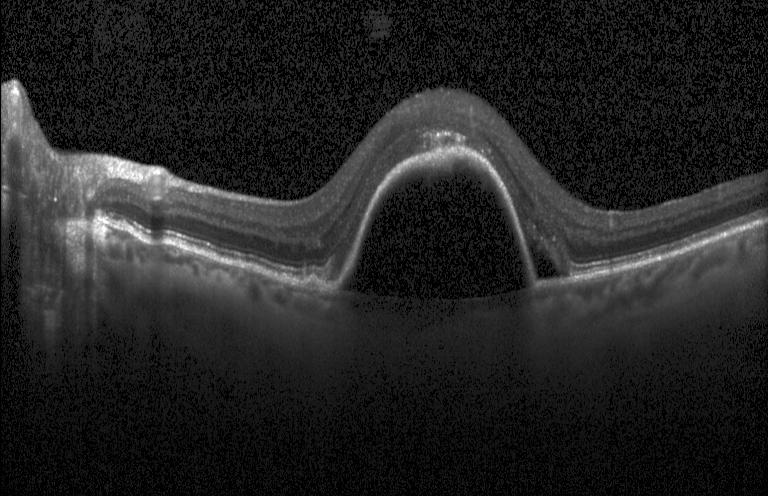
Centered on the fovea, instrument: Heidelberg Spectralis, optical coherence tomography scan.
Dx: choroidal neovascularization (CNV).